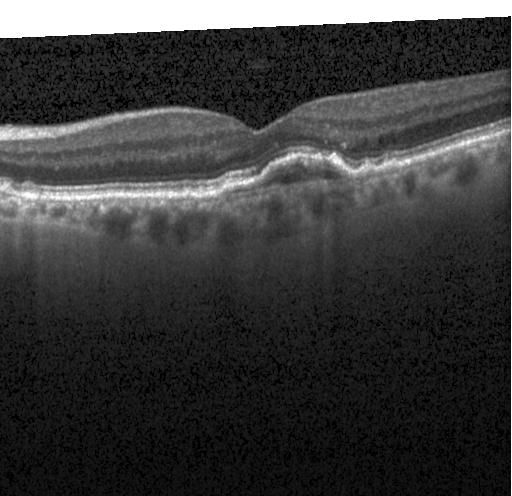
Macular scan; optical coherence tomography B-scan; spectral-domain optical coherence tomography; Heidelberg Spectralis OCT system — Dx: a choroidal neovascular membrane.